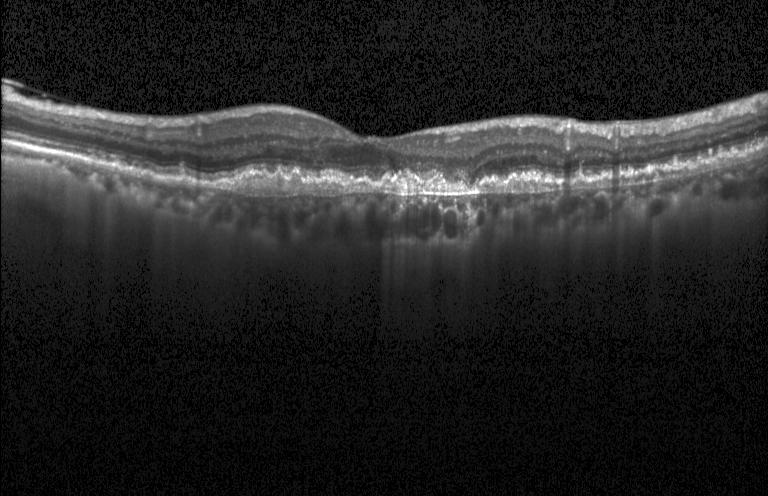 OCT B-scan
Impression: choroidal neovascularization.